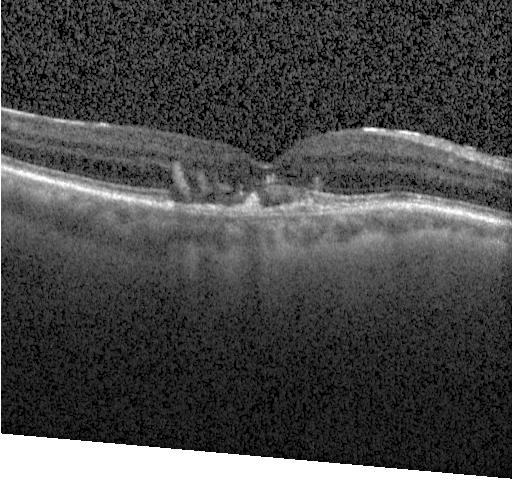
This B-scan demonstrates a choroidal neovascular membrane.